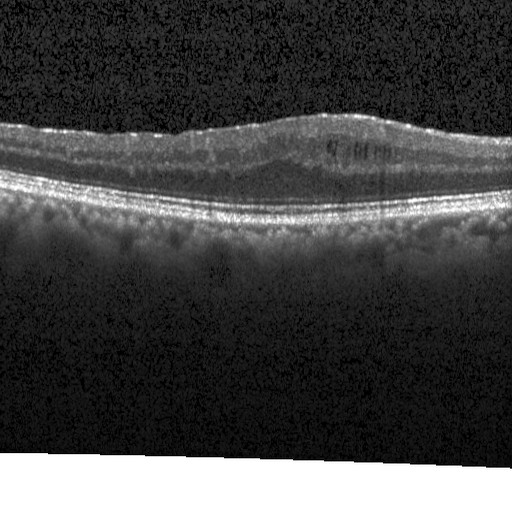 SD-OCT. Heidelberg Spectralis. Horizontal scan through the fovea. OCT B-scan
Impression: diabetic macular edema.